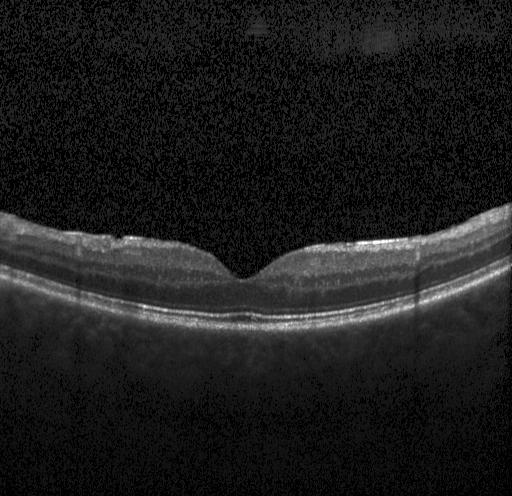

Optical coherence tomography B-scan, spectral-domain optical coherence tomography, Heidelberg Spectralis — This B-scan demonstrates neither choroidal neovascularization, diabetic macular edema, nor drusen.